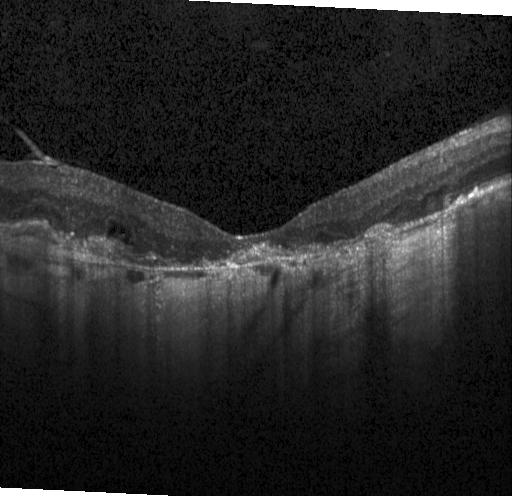
Optical coherence tomography scan, spectral-domain OCT.
Impression: a choroidal neovascular membrane.